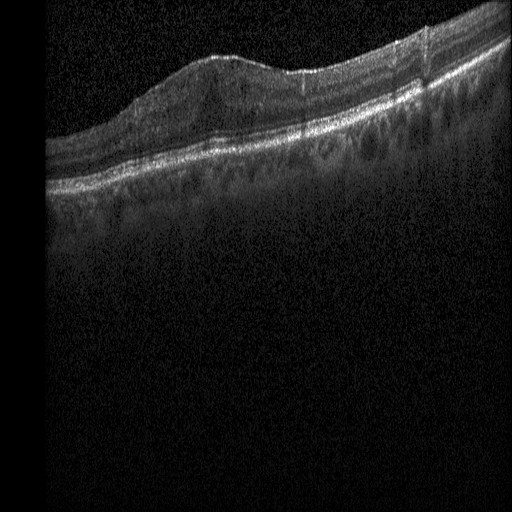
Dx: DME.